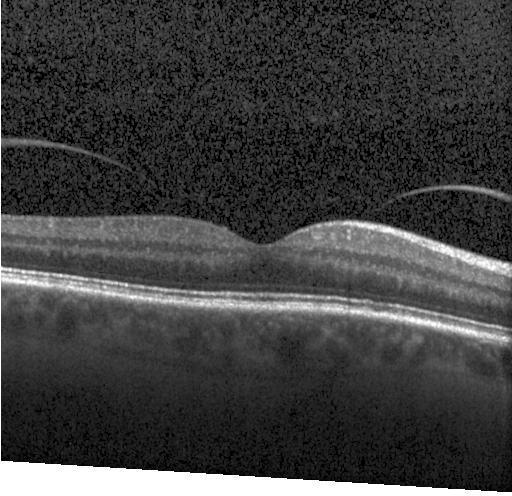

OCT line scan. Acquired on a Heidelberg Spectralis. SD-OCT. Macular scan.
OCT finding: no choroidal neovascularization, no diabetic macular edema, and no drusen.